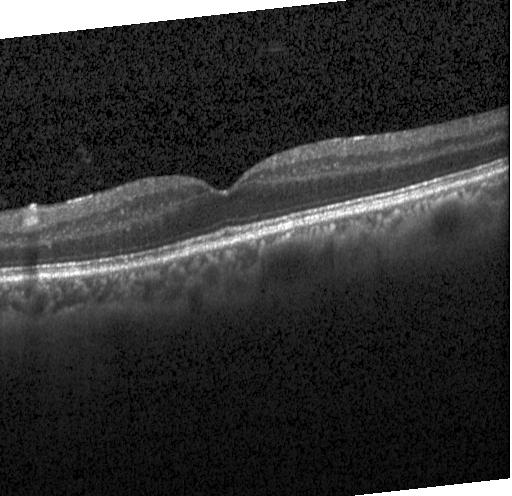

Retinal OCT cross-section, spectral-domain OCT — The scan shows no choroidal neovascularization, no diabetic macular edema, and no drusen.